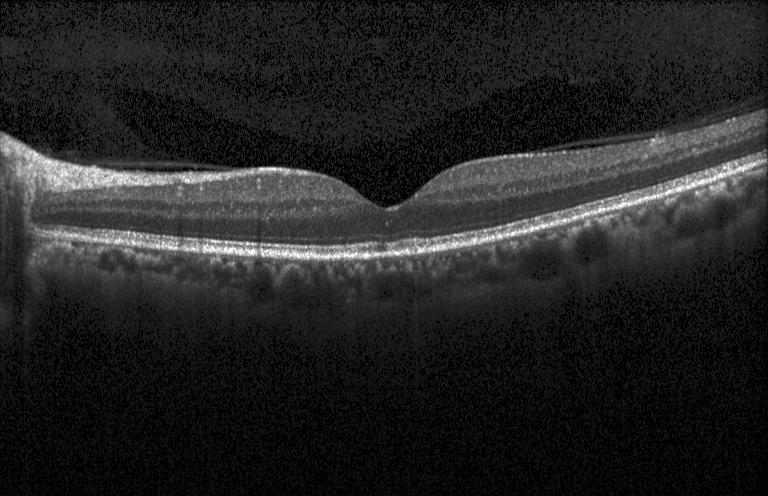 Macular OCT: no evidence of choroidal neovascularization, diabetic macular edema, or drusen.